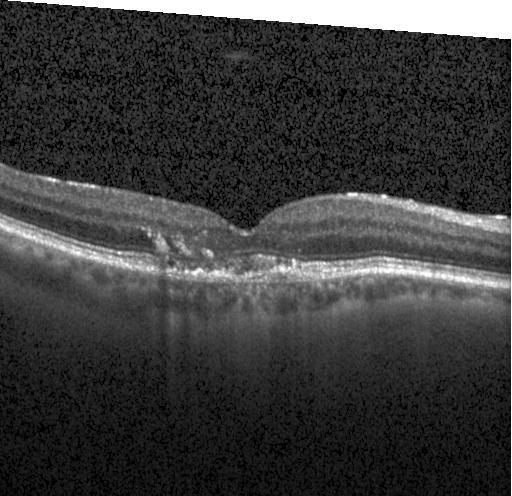 Optical coherence tomography scan, instrument: Heidelberg Spectralis. Finding: a choroidal neovascular membrane.